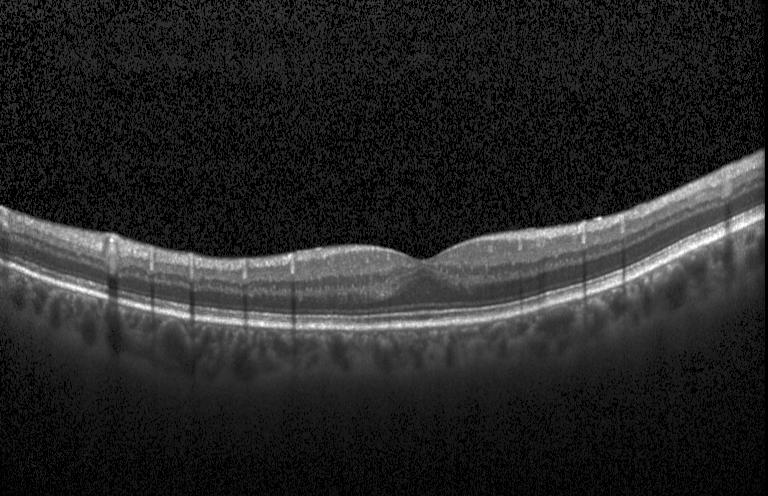 Macular scan · spectral-domain optical coherence tomography · retinal OCT B-scan
Finding: neither CNV, DME, nor drusen.